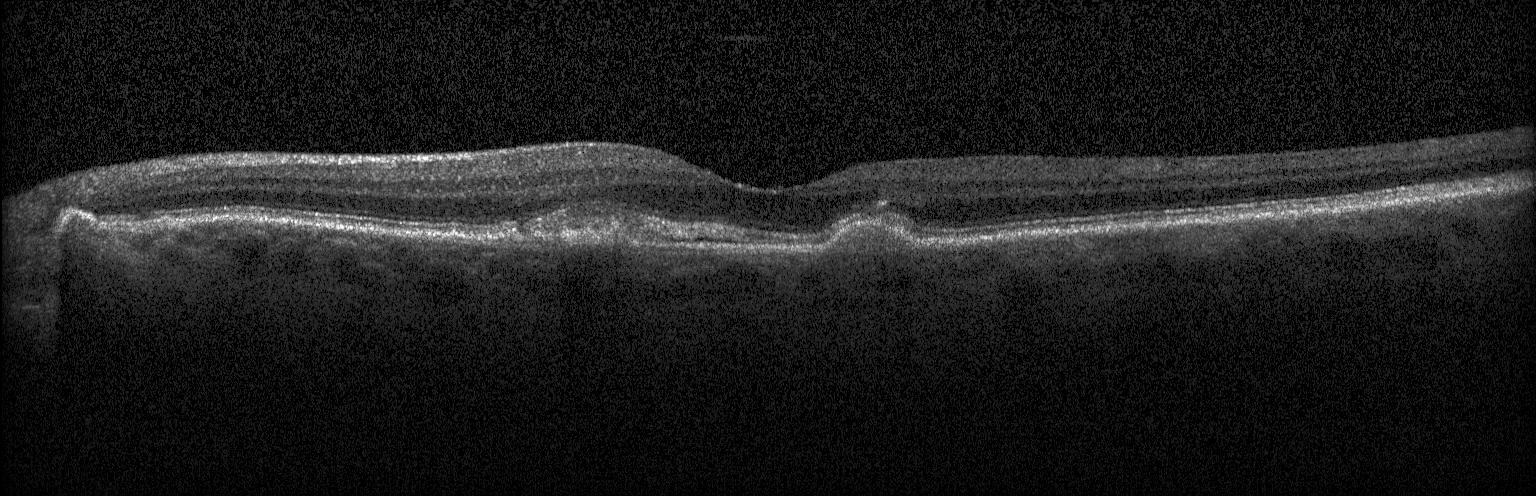
Spectral-domain OCT; retinal OCT B-scan; Heidelberg Spectralis; centered on the fovea.
Diagnosis: CNV.